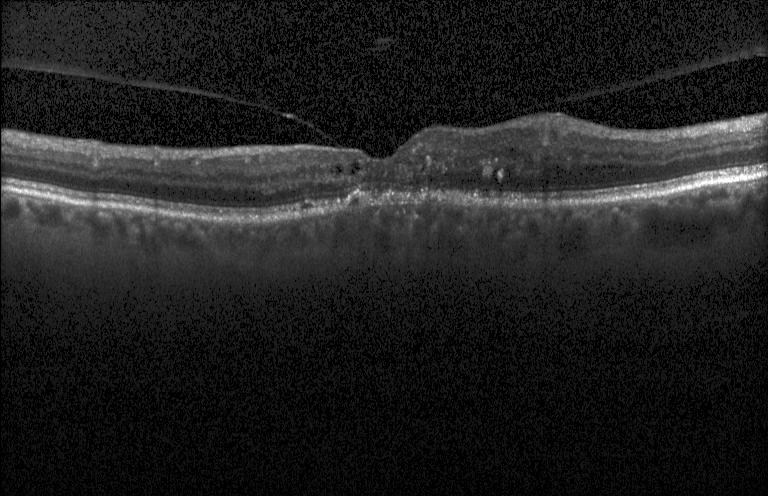
Spectral-domain optical coherence tomography, optical coherence tomography B-scan
Dx: CNV.